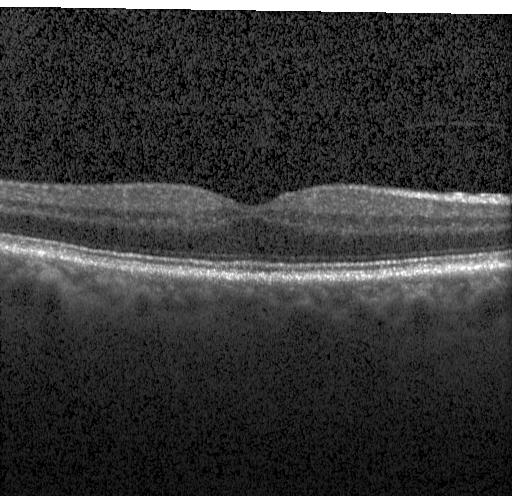

Spectral-domain OCT, OCT B-scan, acquired on a Heidelberg Spectralis — Diagnosis: no evidence of CNV, DME, or drusen.